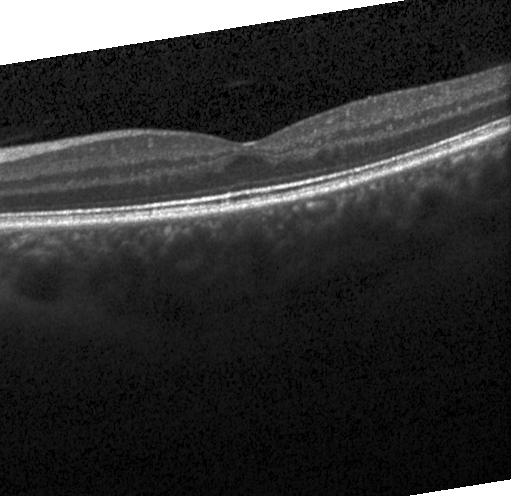

Retinal OCT B-scan
The scan shows no evidence of choroidal neovascularization, diabetic macular edema, or drusen.